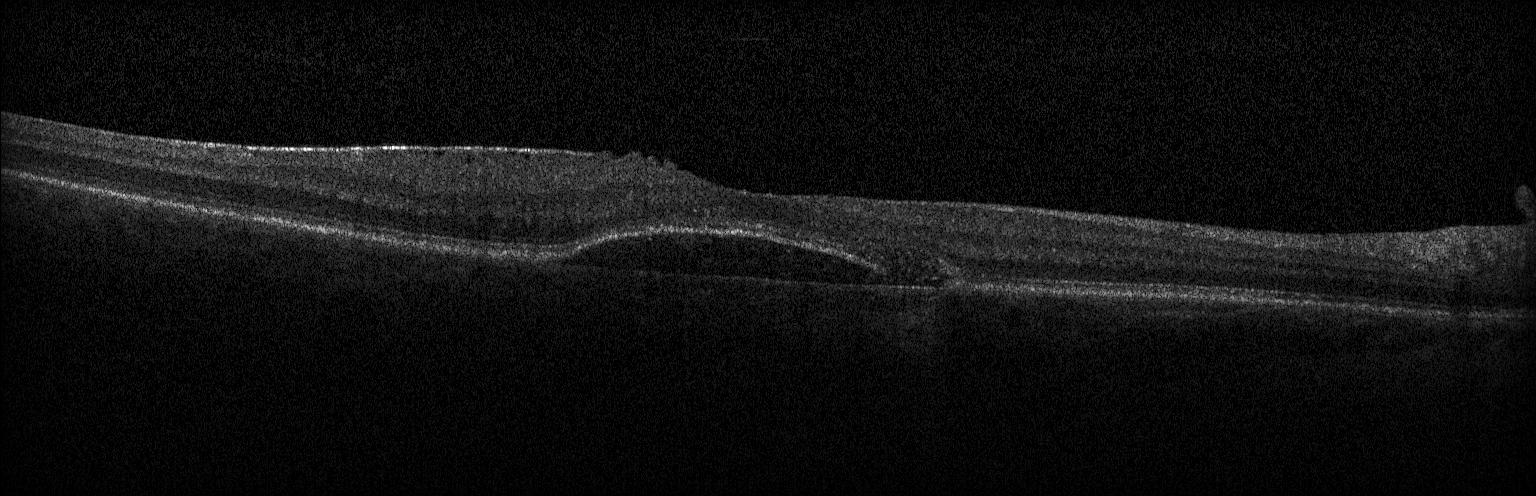
OCT B-scan · Heidelberg Spectralis · SD-OCT · macular scan — The scan shows choroidal neovascularization (CNV).